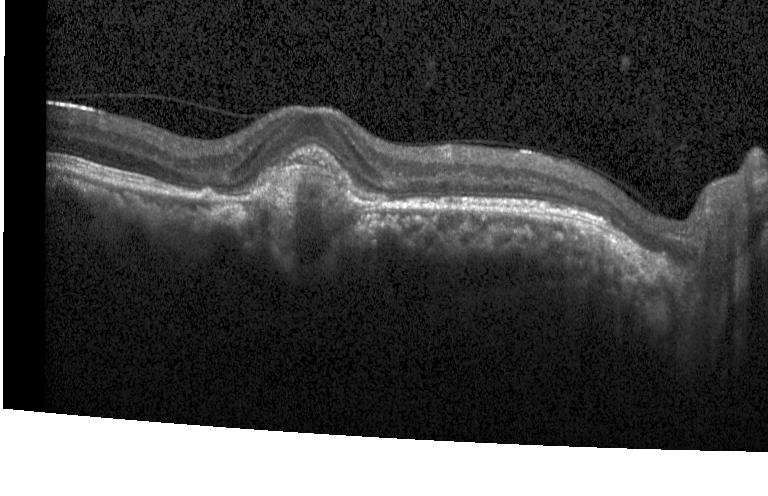 Retinal OCT B-scan — Impression: a choroidal neovascular membrane.